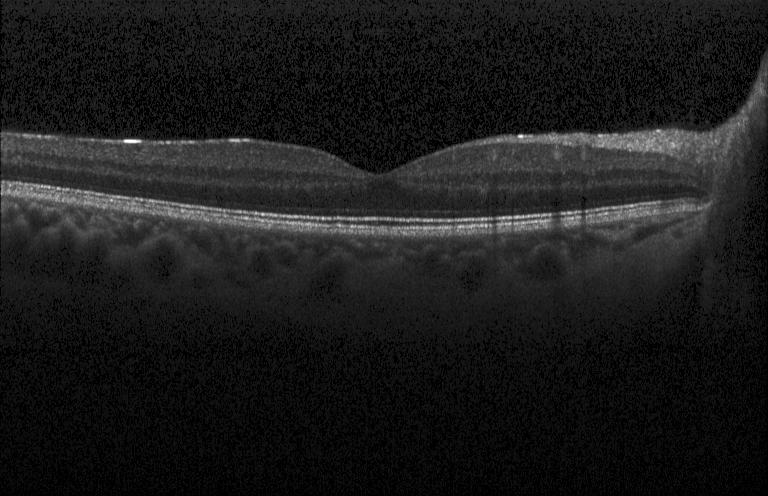

Finding: no evidence of choroidal neovascularization, diabetic macular edema, or drusen.